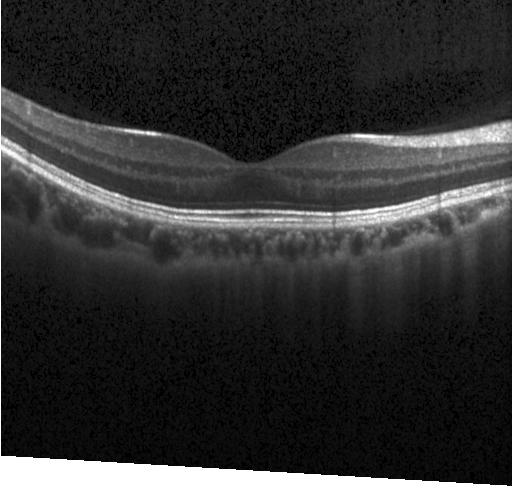
Finding: neither choroidal neovascularization, diabetic macular edema, nor drusen.